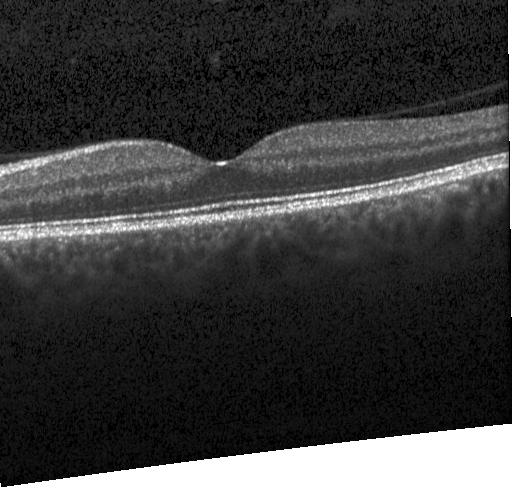

OCT scan showing no choroidal neovascularization, diabetic macular edema, or drusen.